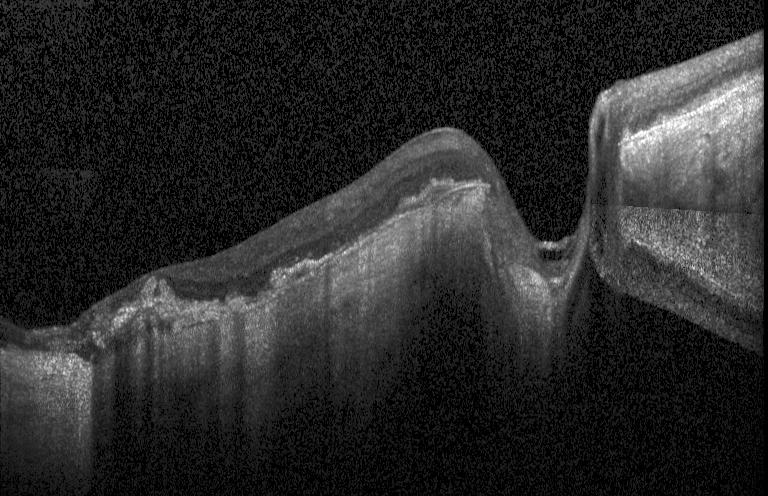

Spectral-domain OCT B-scan: choroidal neovascularization.